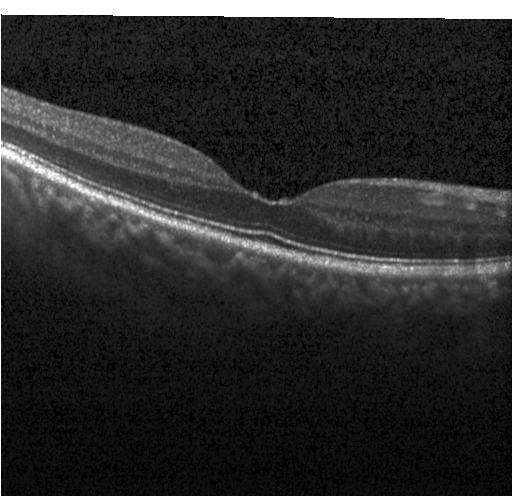

No choroidal neovascularization, diabetic macular edema, or drusen.